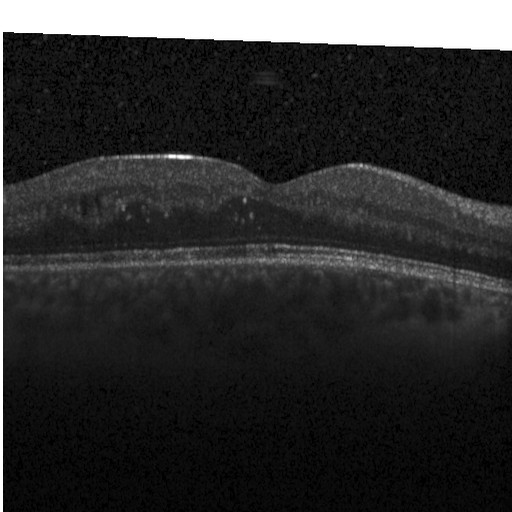

Spectral-domain OCT B-scan: diabetic macular edema.